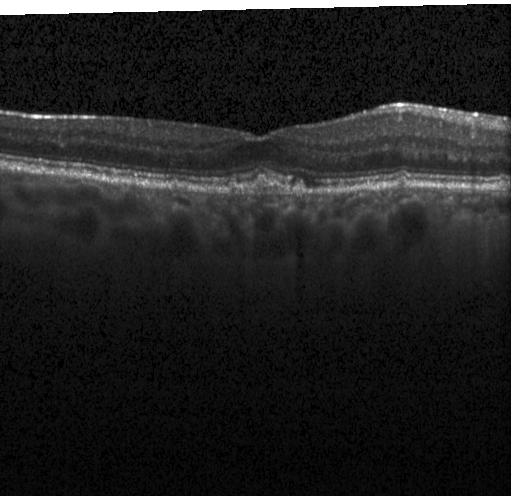
Spectral-domain optical coherence tomography; retinal OCT B-scan; Heidelberg Spectralis; fovea-centered. OCT finding: drusen.